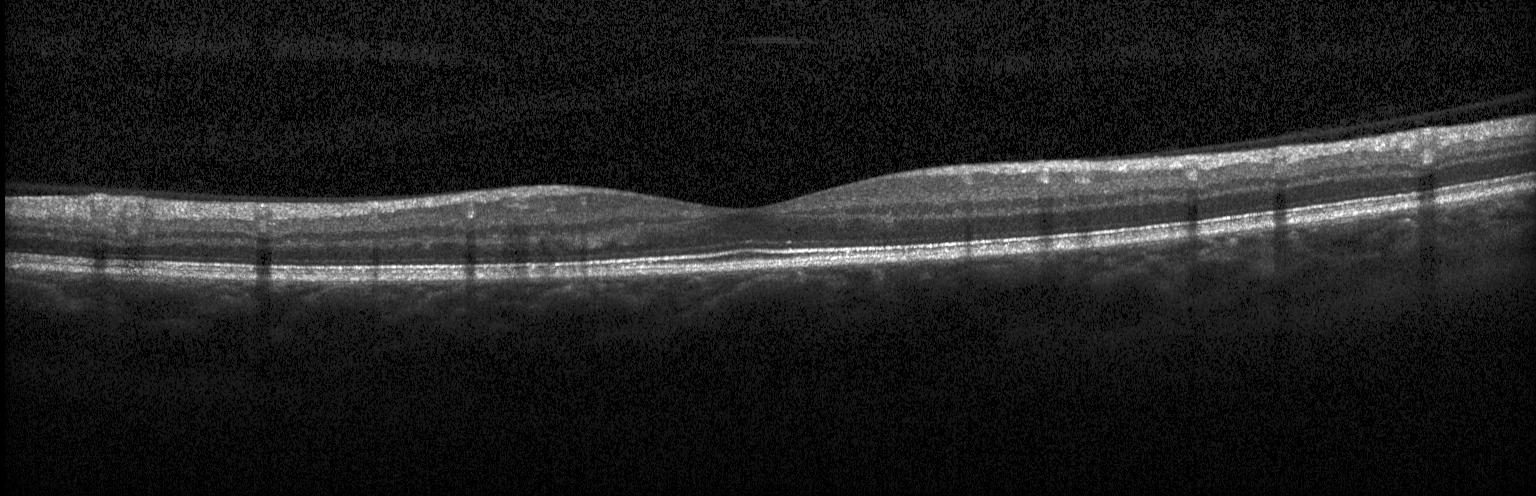

Retinal OCT cross-section; instrument: Heidelberg Spectralis
Diagnosis: no evidence of CNV, DME, or drusen.